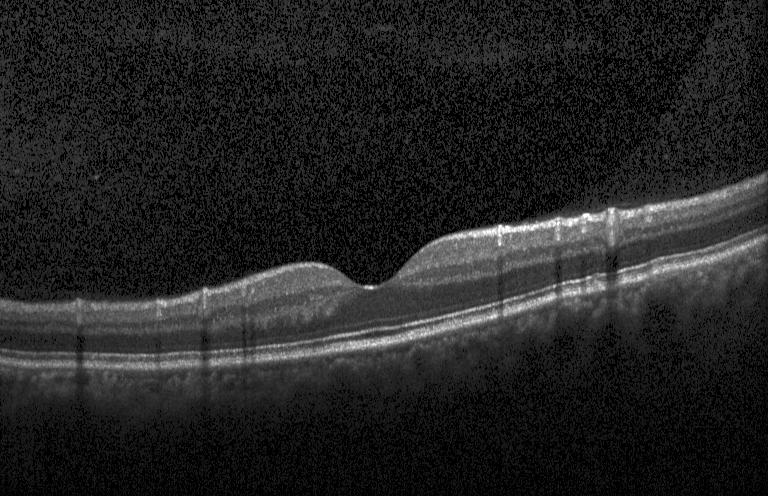 SD-OCT; horizontal scan through the fovea; Heidelberg Spectralis OCT system; optical coherence tomography scan.
This B-scan demonstrates neither CNV, DME, nor drusen.